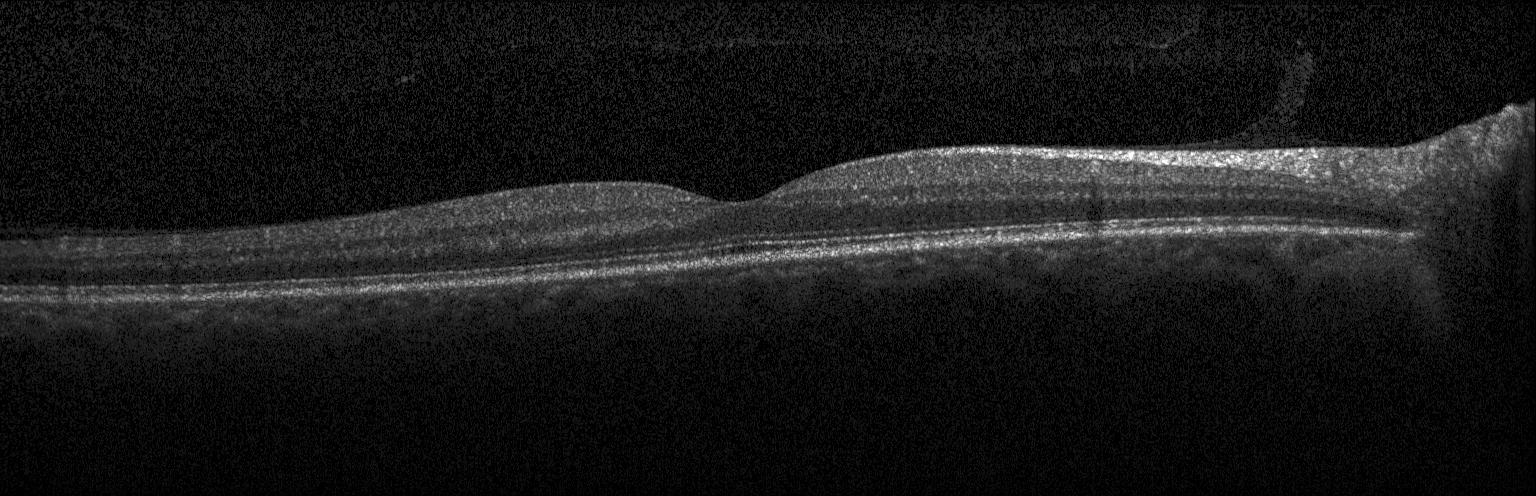

Impression: neither choroidal neovascularization, diabetic macular edema, nor drusen.